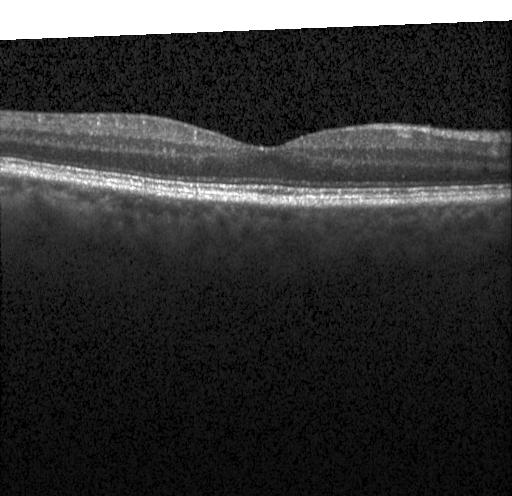 Spectral-domain optical coherence tomography · fovea-centered · retinal OCT cross-section.
Dx: no choroidal neovascularization, diabetic macular edema, or drusen.